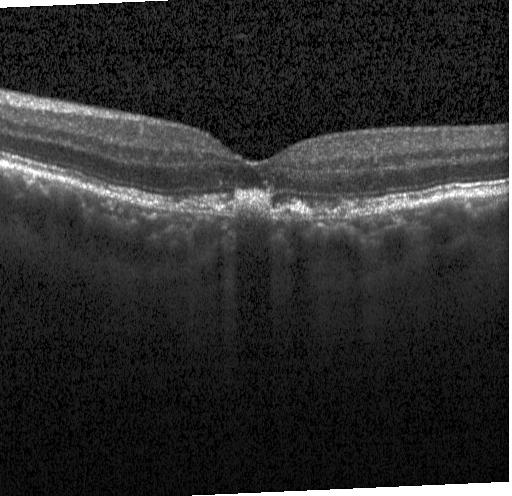

Retinal OCT B-scan — Diagnosis: CNV.